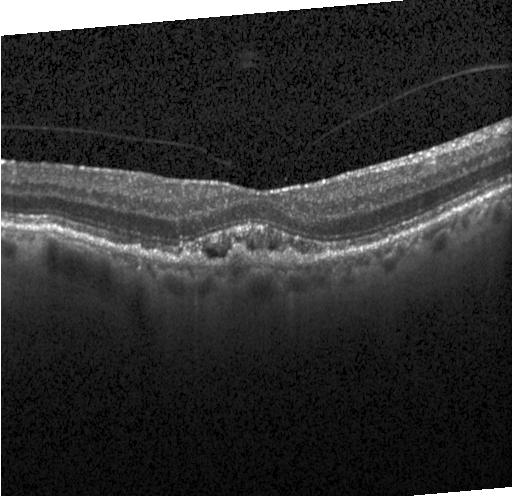
OCT B-scan showing a choroidal neovascular membrane.